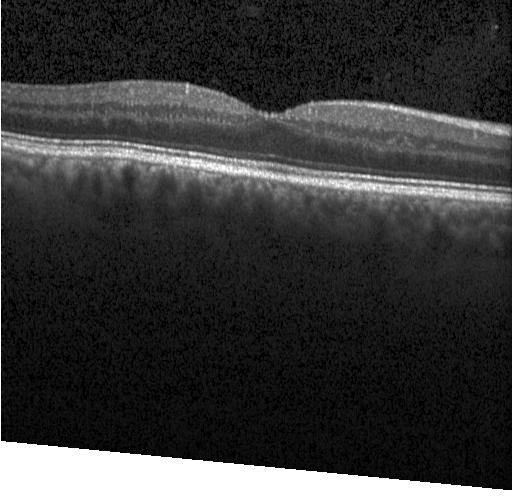
Finding: no evidence of CNV, DME, or drusen.